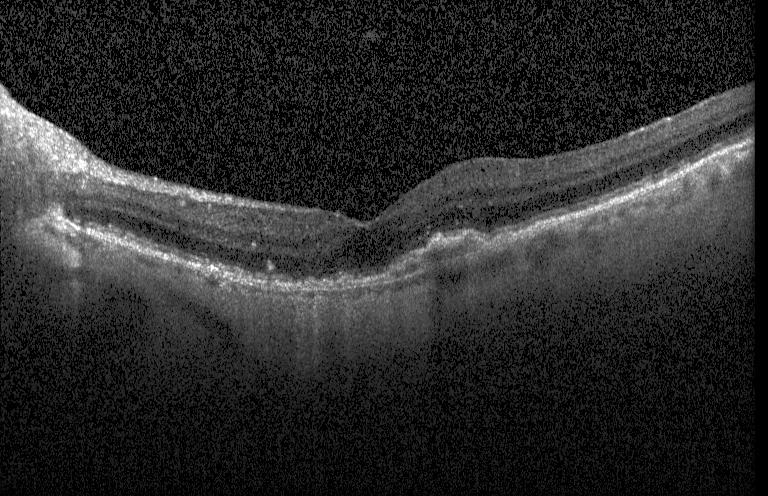

OCT line scan
Assessment: choroidal neovascularization (CNV).